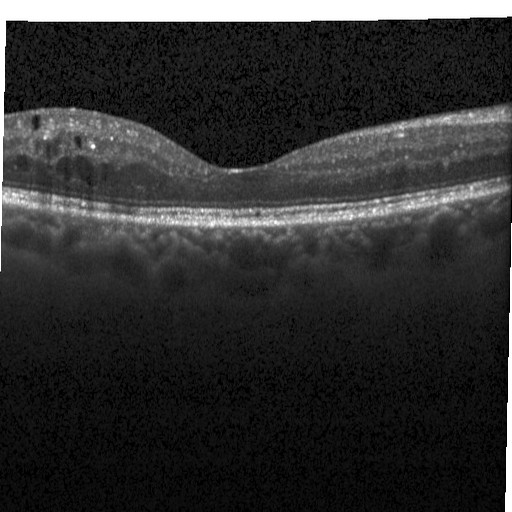

Heidelberg Spectralis OCT system · spectral-domain optical coherence tomography · OCT B-scan.
The scan shows DME.